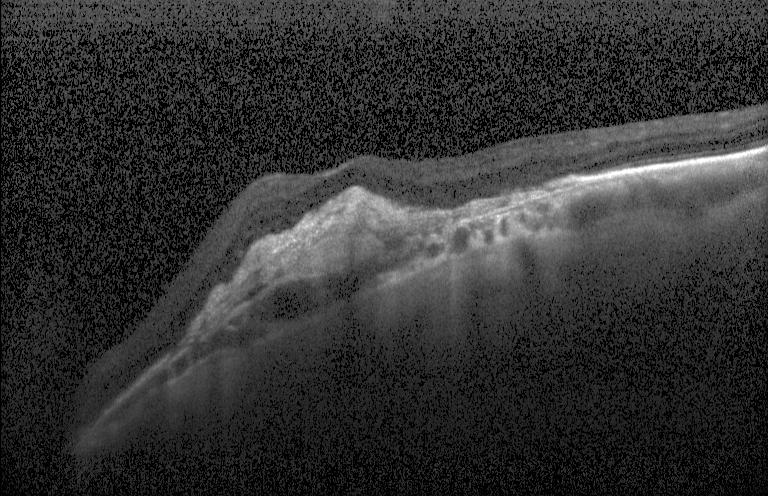 Retinal OCT cross-section showing choroidal neovascularization.